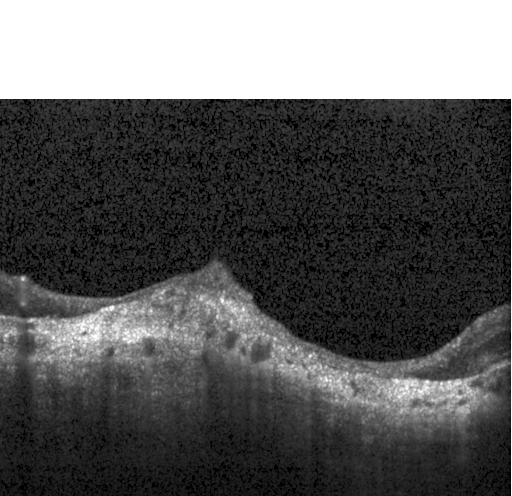
Macular OCT demonstrating choroidal neovascularization.